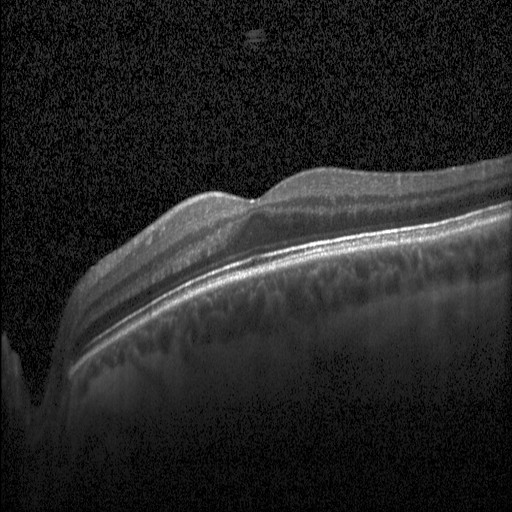 Optical coherence tomography B-scan.
Impression: diabetic macular edema (DME).